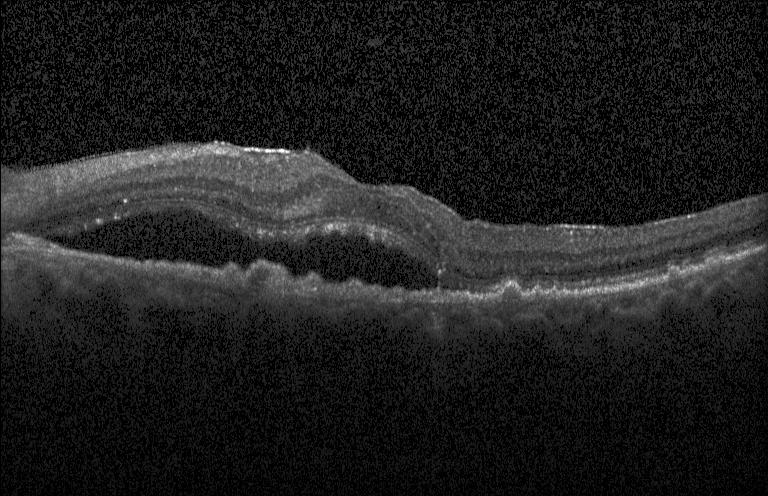
Optical coherence tomography B-scan. OCT finding: choroidal neovascularization (CNV).